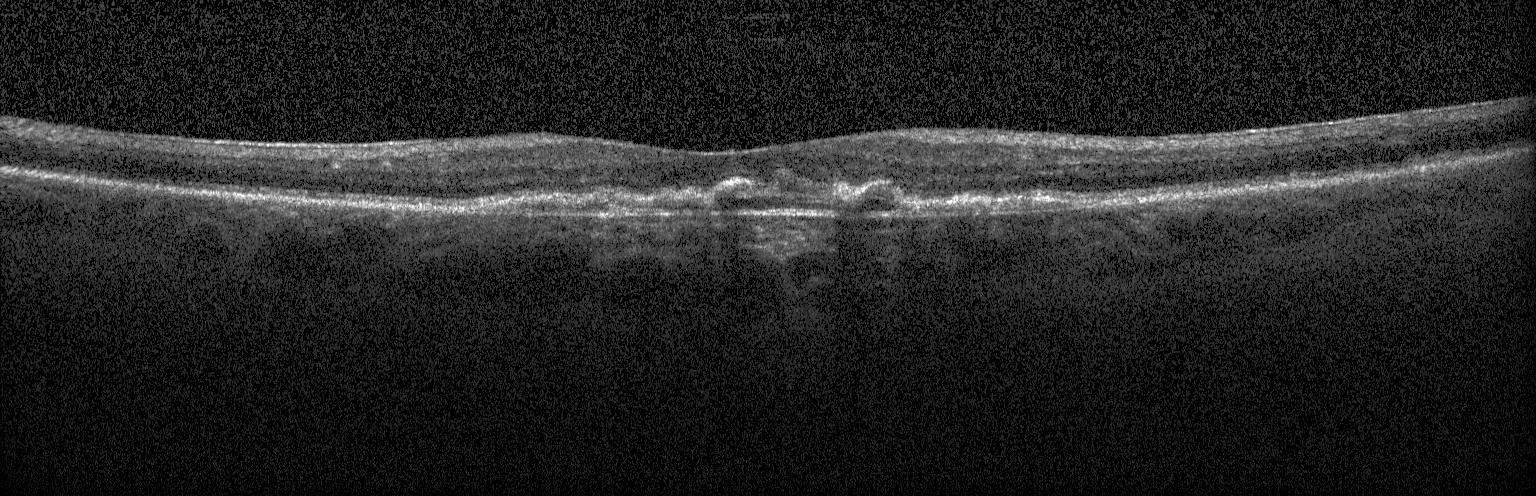

Spectral-domain OCT; OCT B-scan; Heidelberg Spectralis OCT system.
Finding: choroidal neovascularization (CNV).